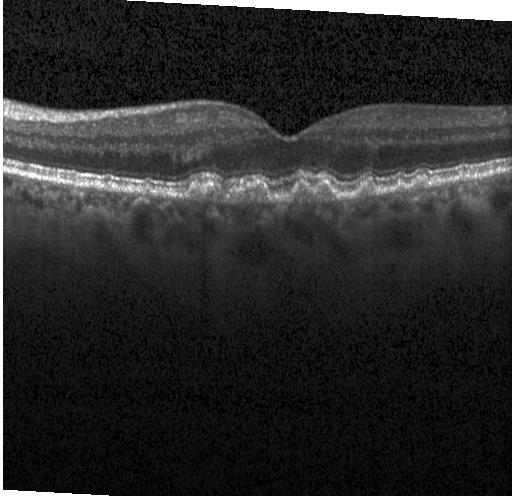 Finding: multiple drusen.